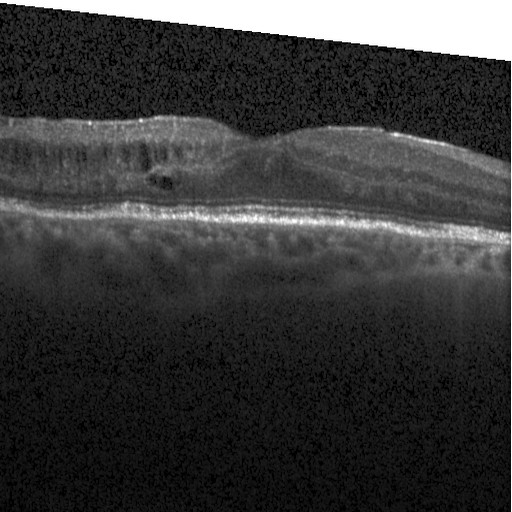 OCT B-scan
Diagnosis: DME.